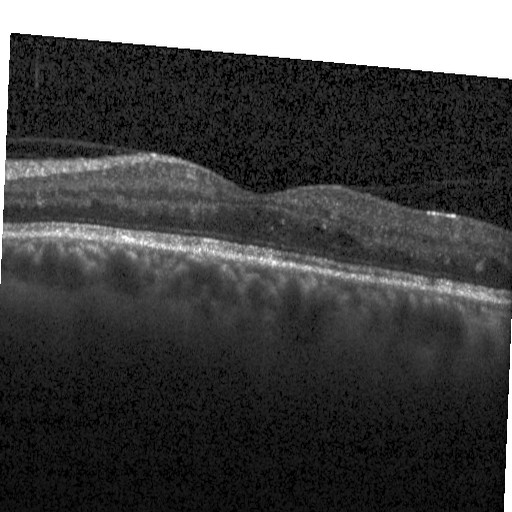 The scan shows diabetic macular edema.